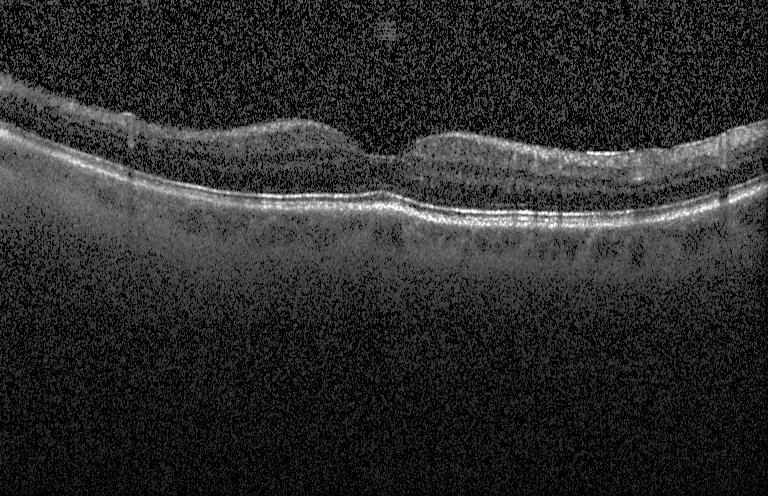
Dx: no evidence of CNV, DME, or drusen.